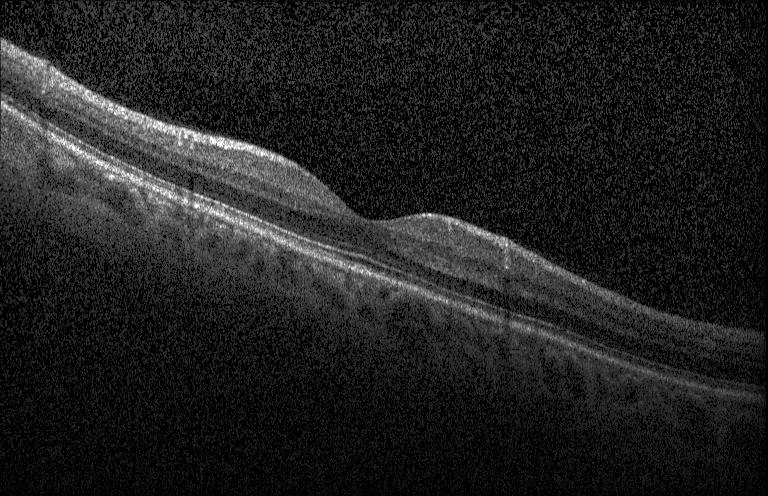 Acquired on a Heidelberg Spectralis; optical coherence tomography B-scan
Assessment: neither CNV, DME, nor drusen.